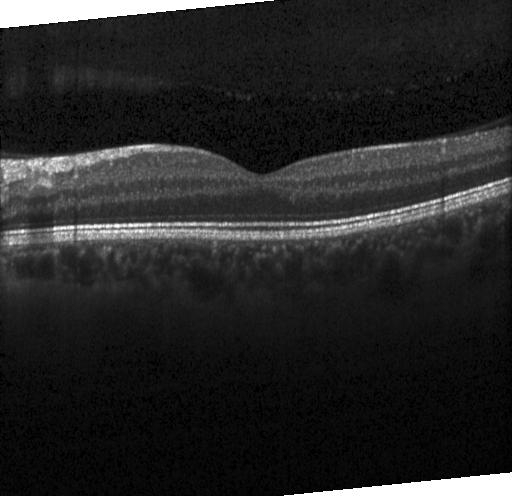
Retinal OCT B-scan, horizontal scan through the fovea, spectral-domain OCT, acquired on a Heidelberg Spectralis.
Finding: no evidence of choroidal neovascularization, diabetic macular edema, or drusen.